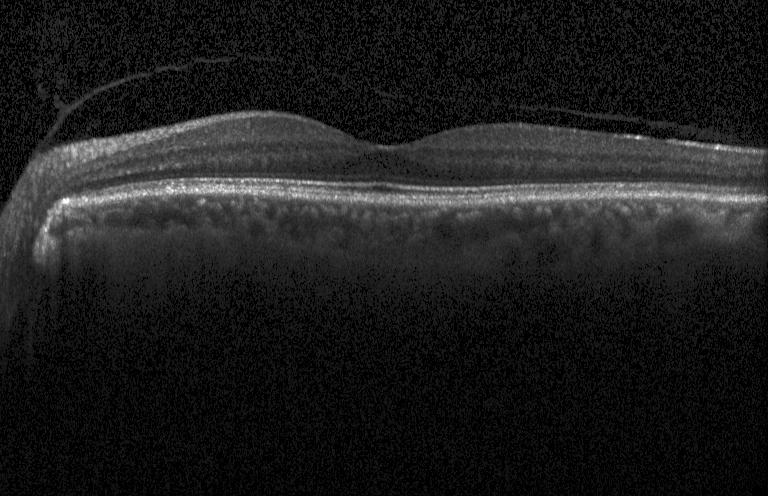

Optical coherence tomography B-scan. Spectral-domain optical coherence tomography. Acquired on a Heidelberg Spectralis. Finding: no choroidal neovascularization, no diabetic macular edema, and no drusen.